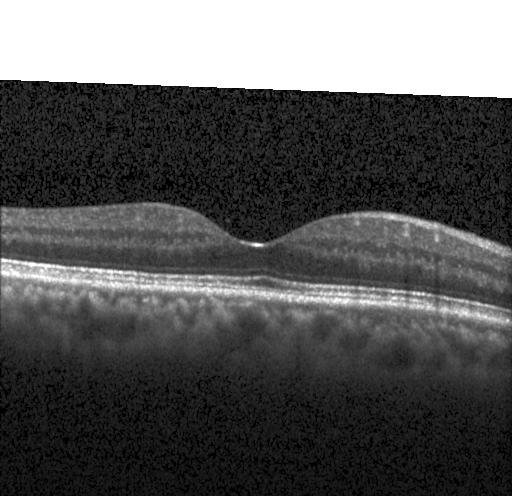

OCT B-scan. SD-OCT
The scan shows neither choroidal neovascularization, diabetic macular edema, nor drusen.